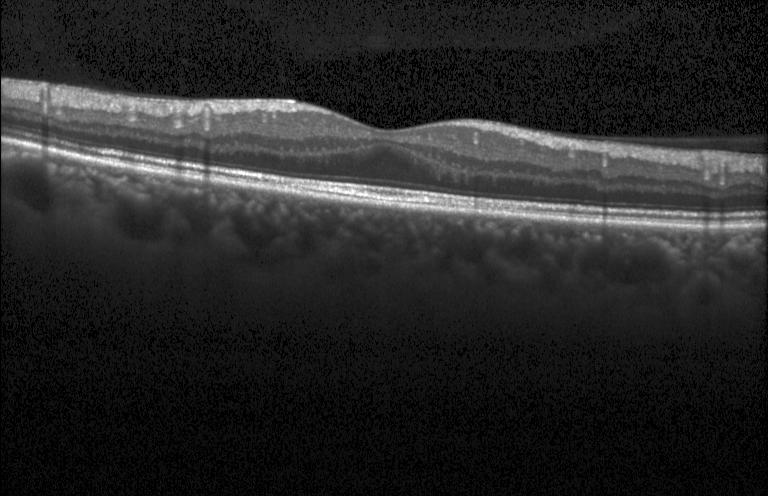
Spectral-domain optical coherence tomography. Macular scan. Retinal OCT cross-section
Macular OCT: neither CNV, DME, nor drusen.